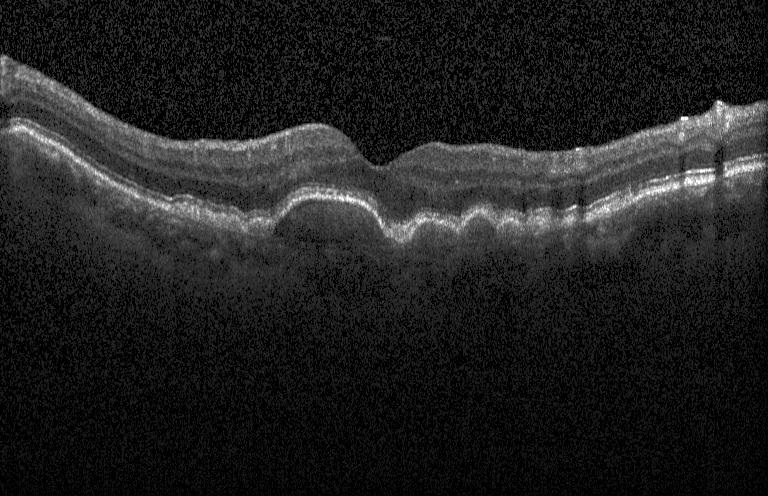

Acquired on a Heidelberg Spectralis. Optical coherence tomography B-scan.
Diagnosis: drusen.